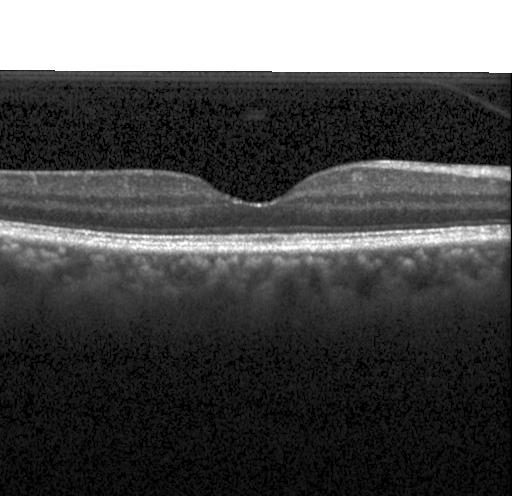
Finding: no CNV, DME, or drusen.